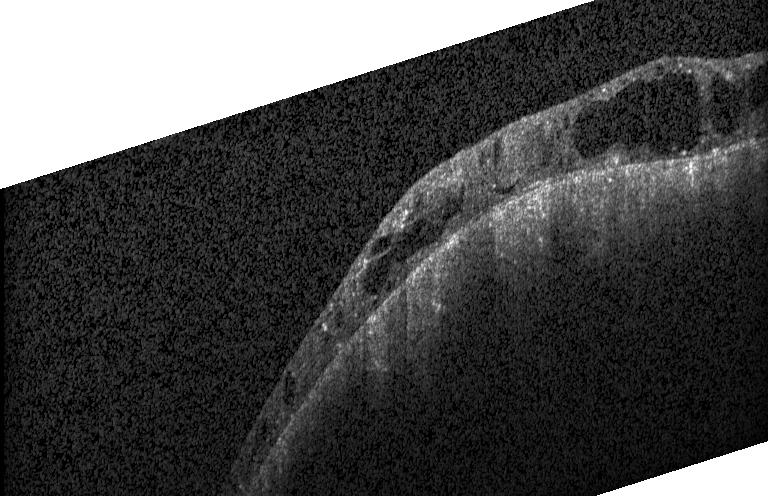

Optical coherence tomography scan, centered on the fovea. Diagnosis: DME.